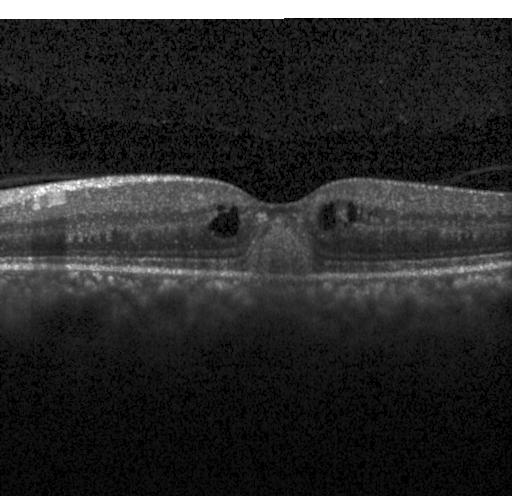
Macular OCT demonstrating a choroidal neovascular membrane.